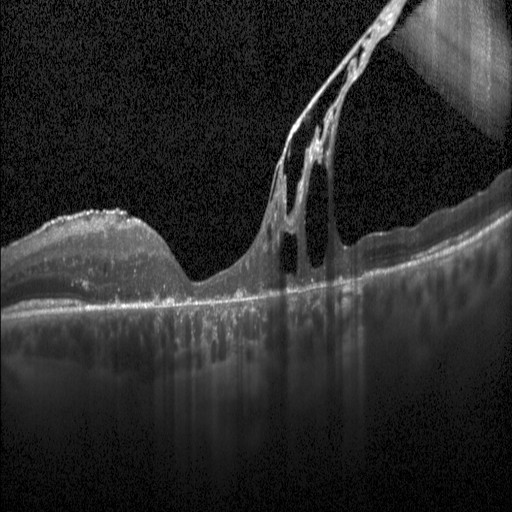
Spectral-domain optical coherence tomography; through the macula; retinal OCT B-scan; acquired on a Heidelberg Spectralis — Diabetic macular edema.